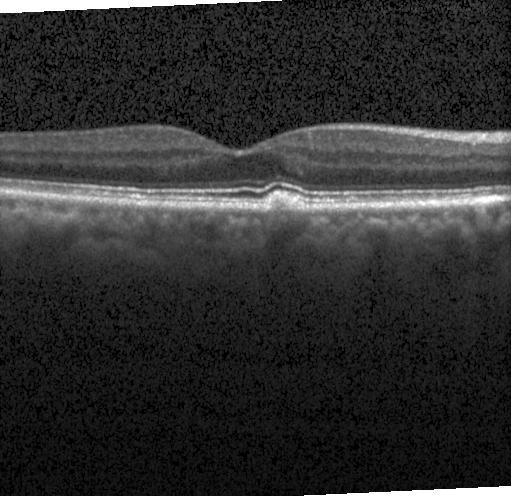

Impression: sub-RPE drusenoid deposits.